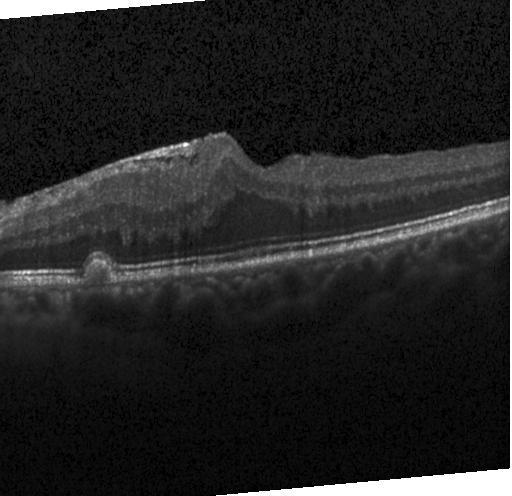

Impression: sub-RPE drusenoid deposits.